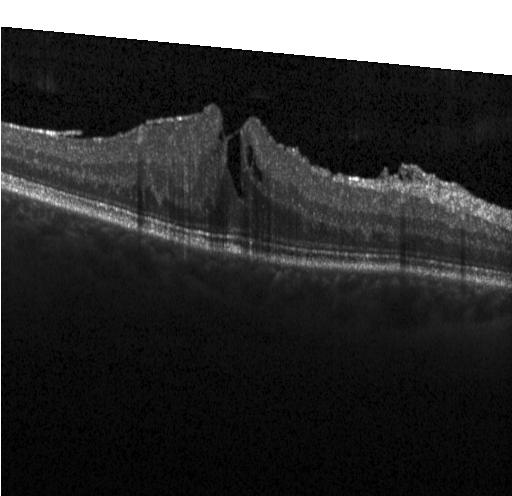 Spectral-domain OCT. OCT B-scan. Heidelberg Spectralis. Impression: diabetic macular edema (DME).